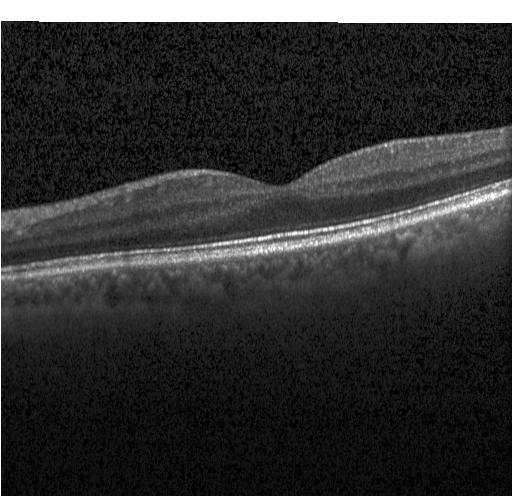

Retinal OCT B-scan; acquired on a Heidelberg Spectralis.
Macular OCT: no choroidal neovascularization, diabetic macular edema, or drusen.